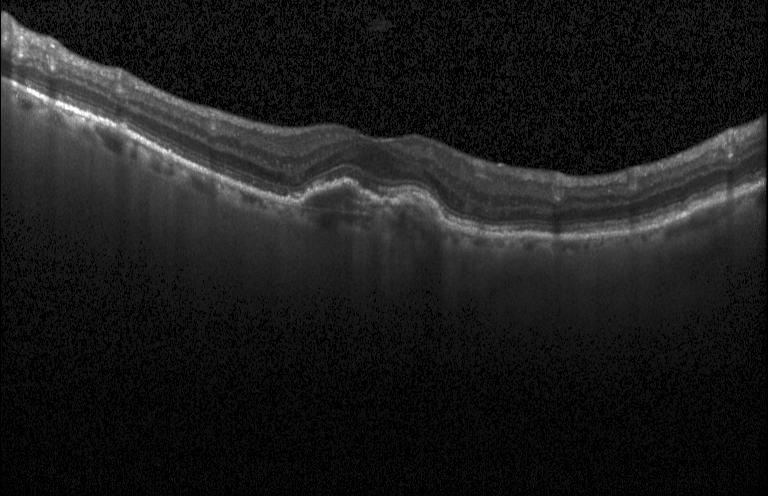

The scan shows a choroidal neovascular membrane.